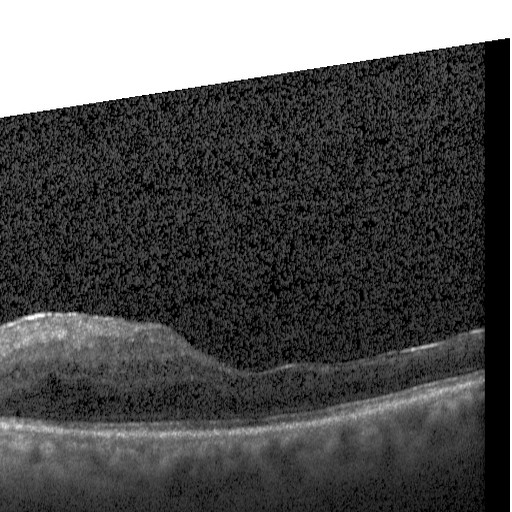 Retinal OCT B-scan — Diabetic macular edema (DME).